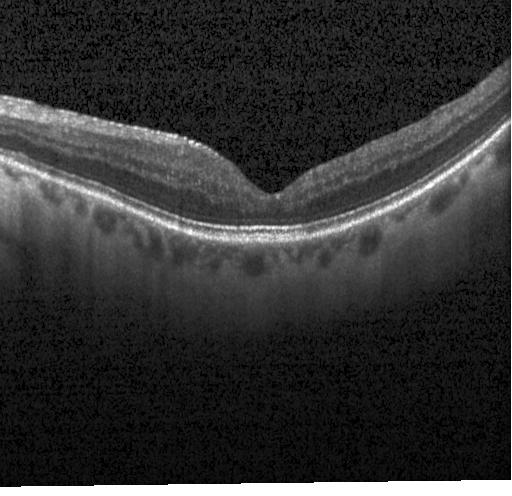
OCT finding: neither choroidal neovascularization, diabetic macular edema, nor drusen.